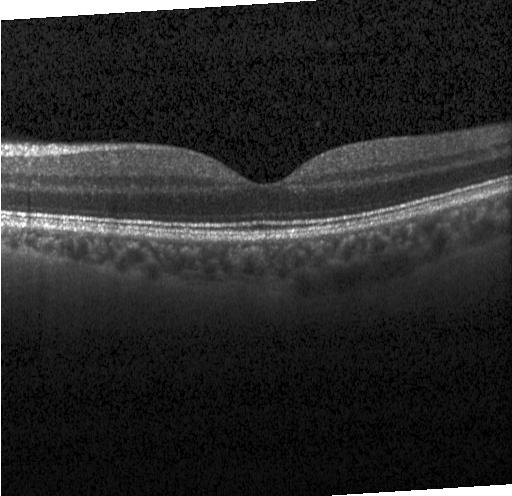

OCT B-scan.
OCT finding: neither choroidal neovascularization, diabetic macular edema, nor drusen.